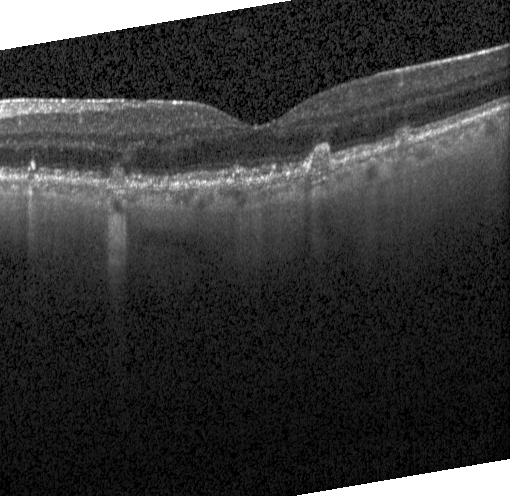 OCT finding: sub-RPE drusenoid deposits.